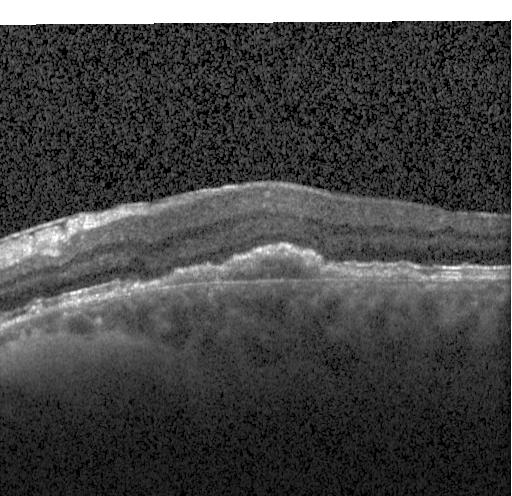

Choroidal neovascularization (CNV).